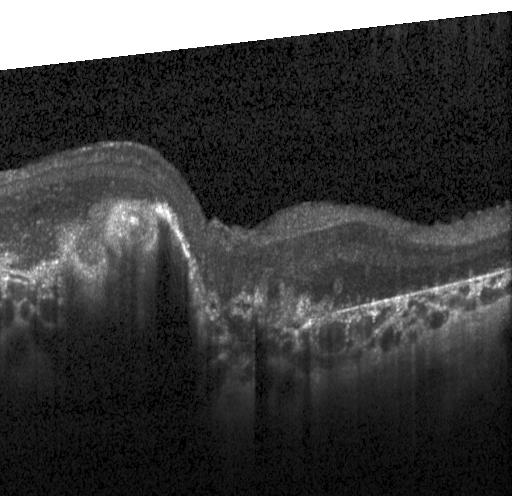

Acquired on a Heidelberg Spectralis. Through the macula. SD-OCT. OCT B-scan. The scan shows choroidal neovascularization (CNV).